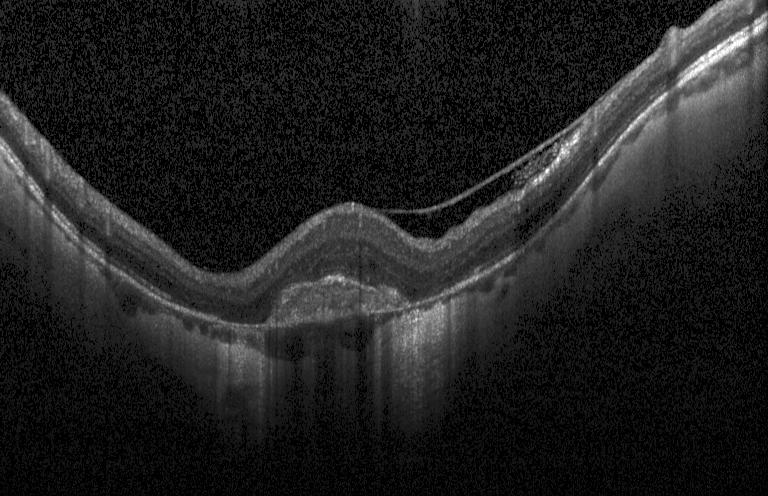 Retinal OCT cross-section.
Macular OCT: a choroidal neovascular membrane.